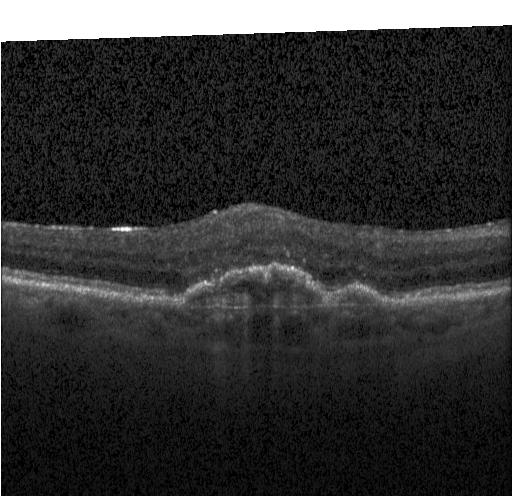
Optical coherence tomography B-scan — Assessment: choroidal neovascularization (CNV).